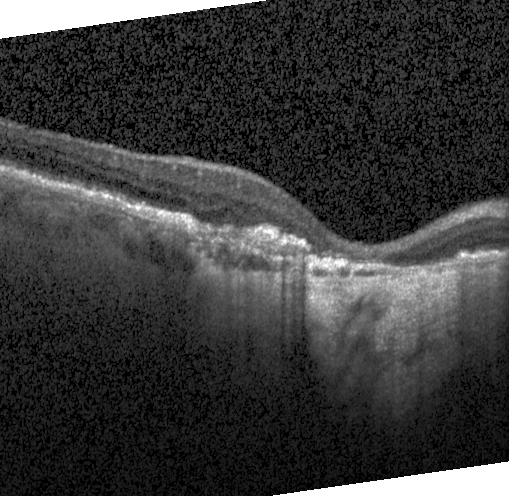

Retinal OCT cross-section — A choroidal neovascular membrane.